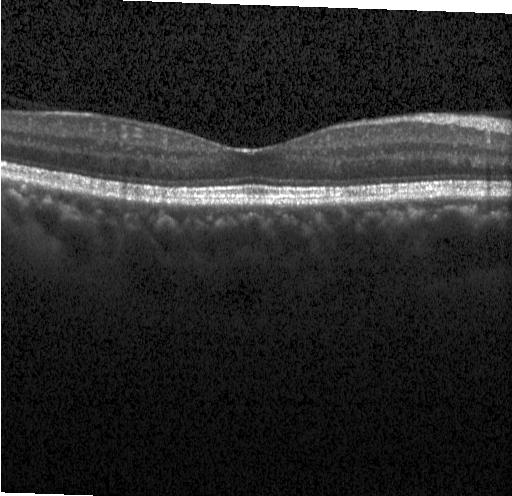 Acquired on a Heidelberg Spectralis · retinal OCT cross-section · spectral-domain OCT · macular scan
The scan shows no choroidal neovascularization, no diabetic macular edema, and no drusen.